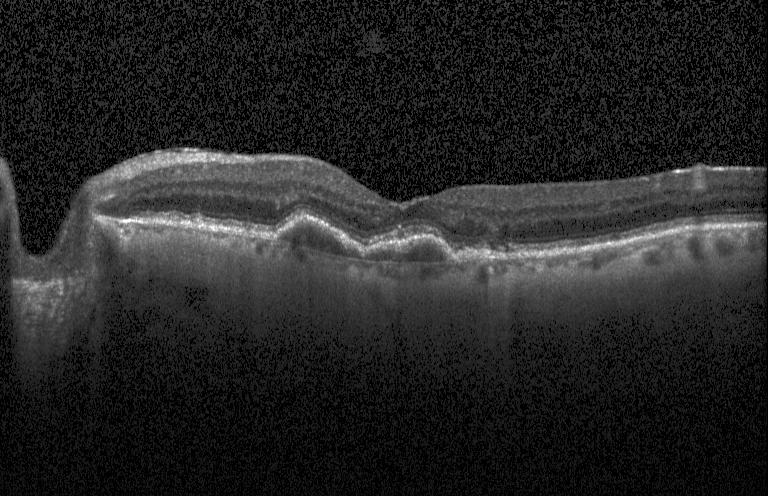
Retinal OCT B-scan.
Impression: a choroidal neovascular membrane.